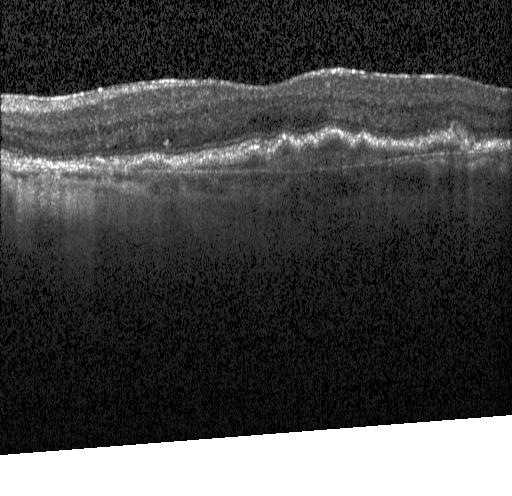 Optical coherence tomography scan; fovea-centered; spectral-domain optical coherence tomography.
Impression: choroidal neovascularization (CNV).